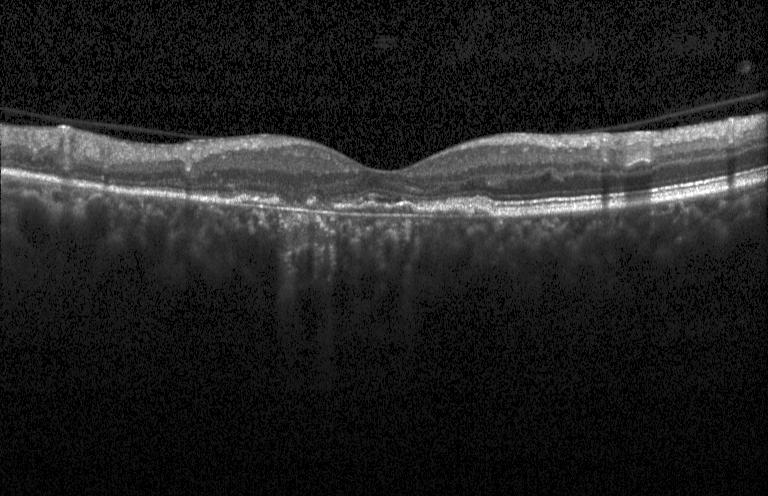

SD-OCT. Heidelberg Spectralis OCT system. Macular scan. Retinal OCT cross-section — Macular OCT: a choroidal neovascular membrane.